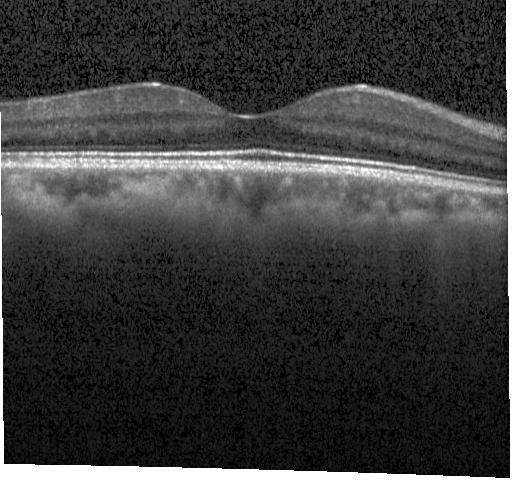
Spectral-domain OCT, OCT B-scan, Heidelberg Spectralis OCT system
Finding: no choroidal neovascularization, diabetic macular edema, or drusen.